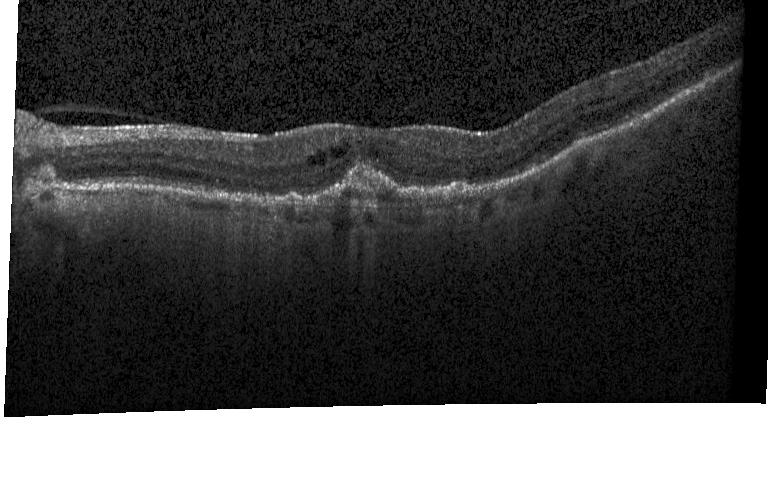 Horizontal scan through the fovea, retinal OCT cross-section.
Assessment: a choroidal neovascular membrane.